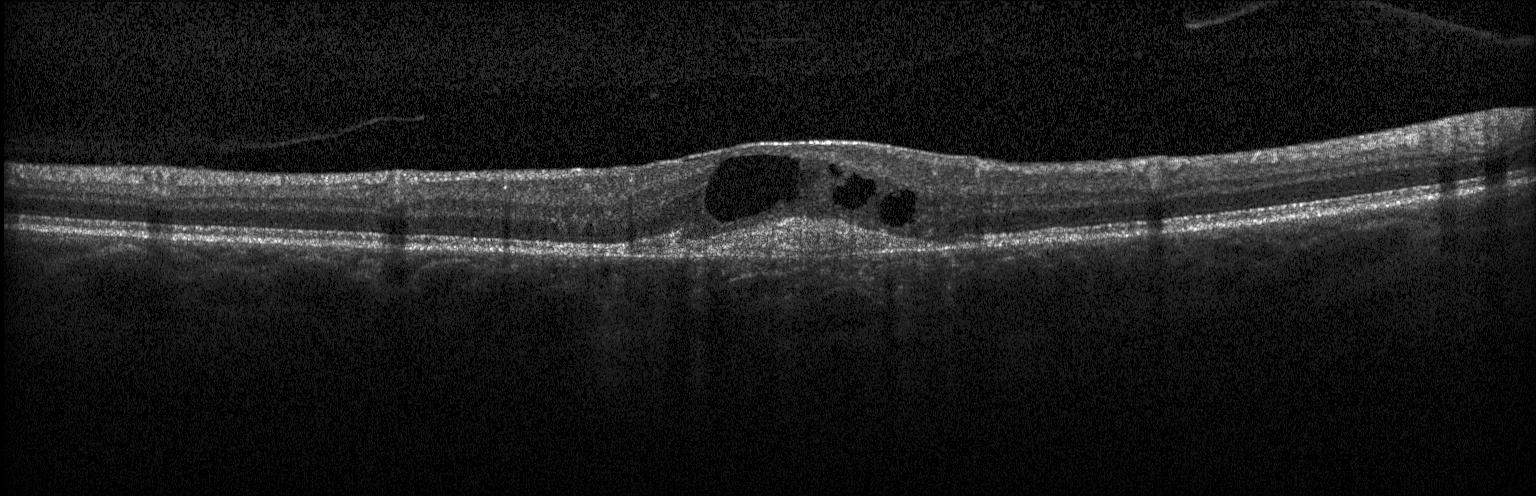

Optical coherence tomography B-scan · acquired on a Heidelberg Spectralis.
Impression: choroidal neovascularization (CNV).